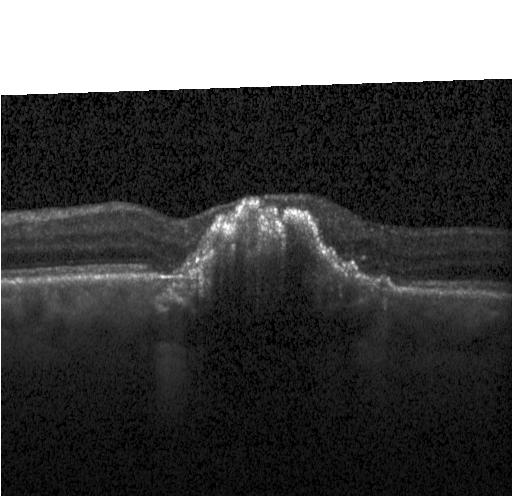 Macular OCT: a choroidal neovascular membrane.